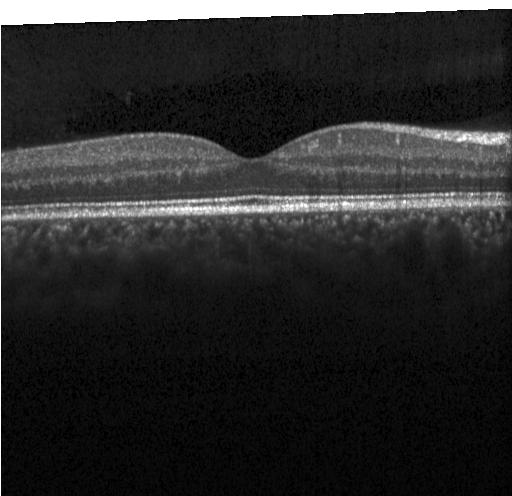

Finding: no CNV, DME, or drusen.